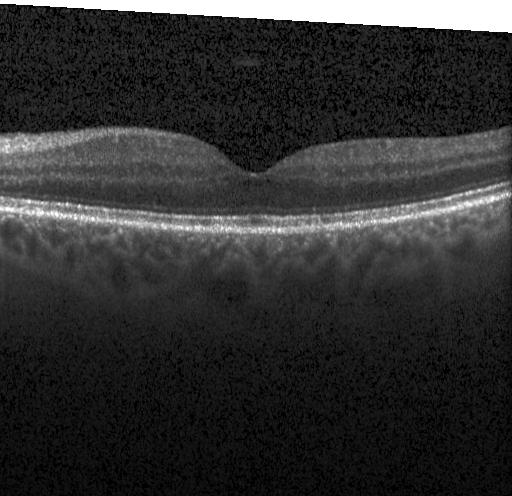 Heidelberg Spectralis OCT system · optical coherence tomography B-scan
This B-scan demonstrates neither choroidal neovascularization, diabetic macular edema, nor drusen.